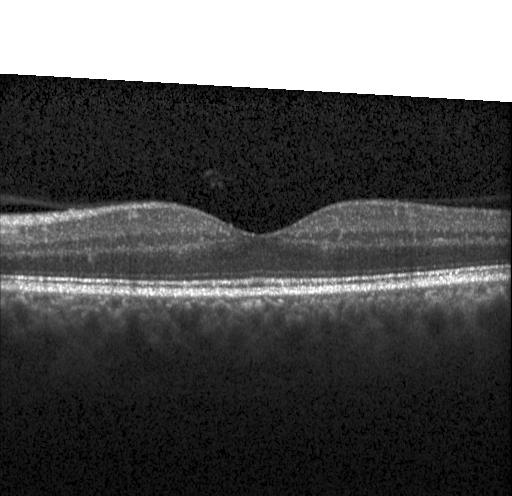 Retinal OCT B-scan — Diagnosis: neither CNV, DME, nor drusen.